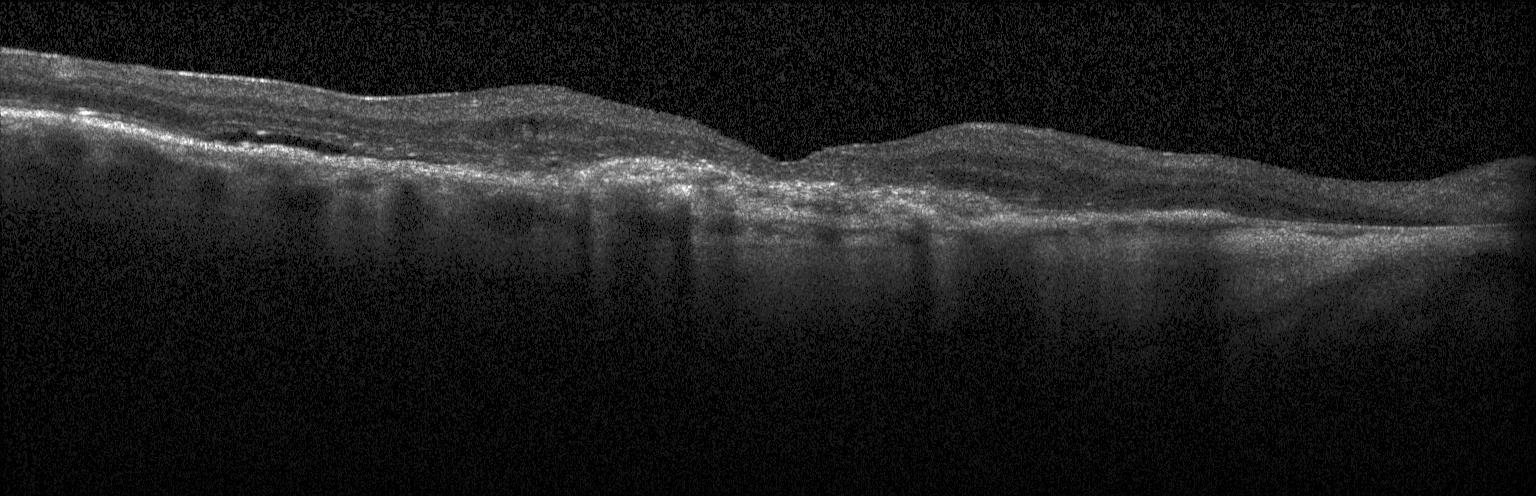 Macular OCT: a choroidal neovascular membrane.